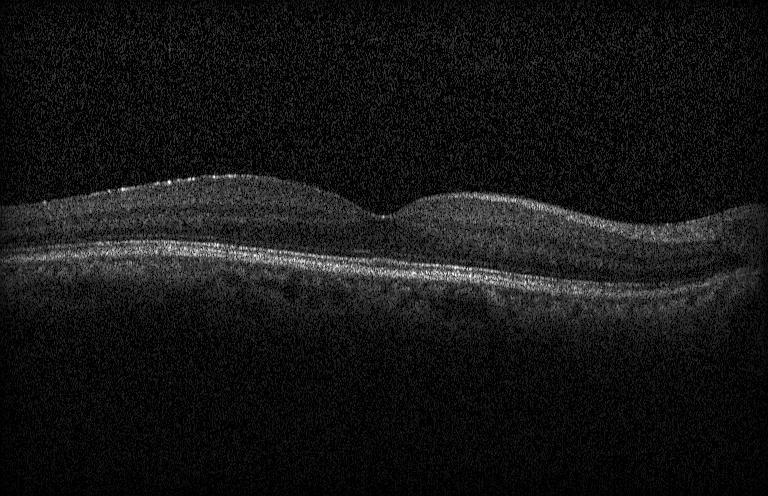 Retinal OCT cross-section showing no choroidal neovascularization, diabetic macular edema, or drusen.